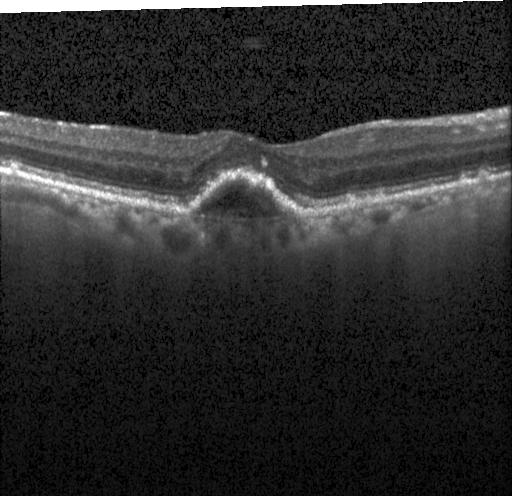
Spectral-domain optical coherence tomography. Retinal OCT B-scan — Macular OCT: choroidal neovascularization (CNV).